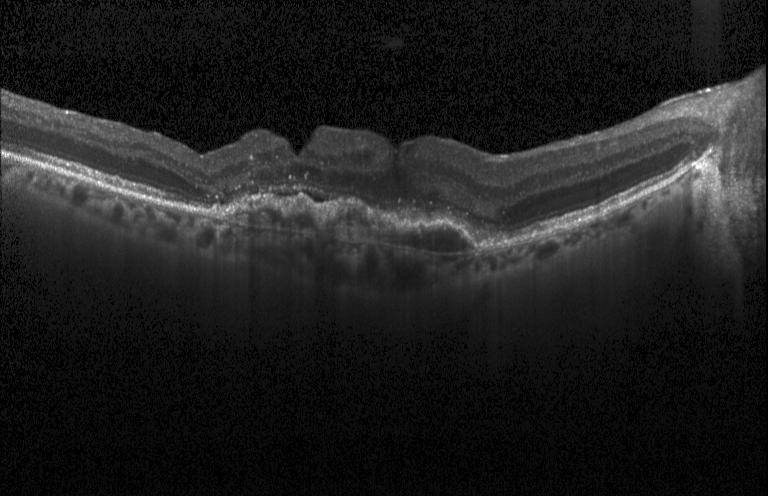
Diagnosis: a choroidal neovascular membrane.